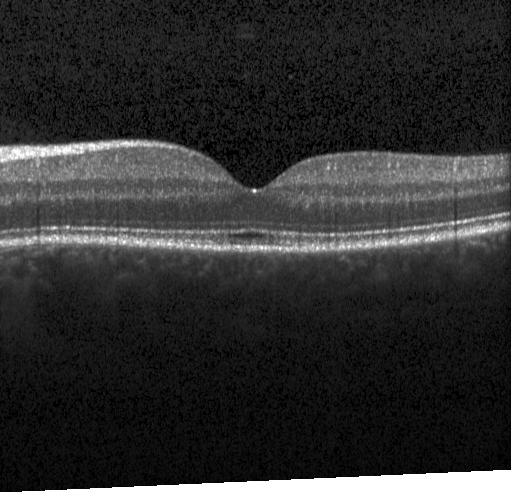
Spectral-domain OCT B-scan: no evidence of choroidal neovascularization, diabetic macular edema, or drusen.